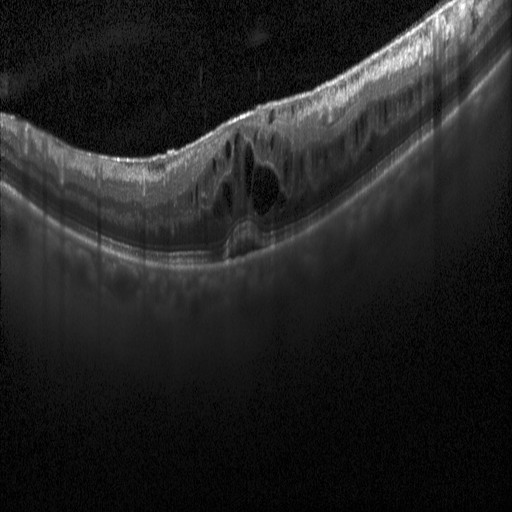

SD-OCT, retinal OCT cross-section. Impression: diabetic macular edema (DME).